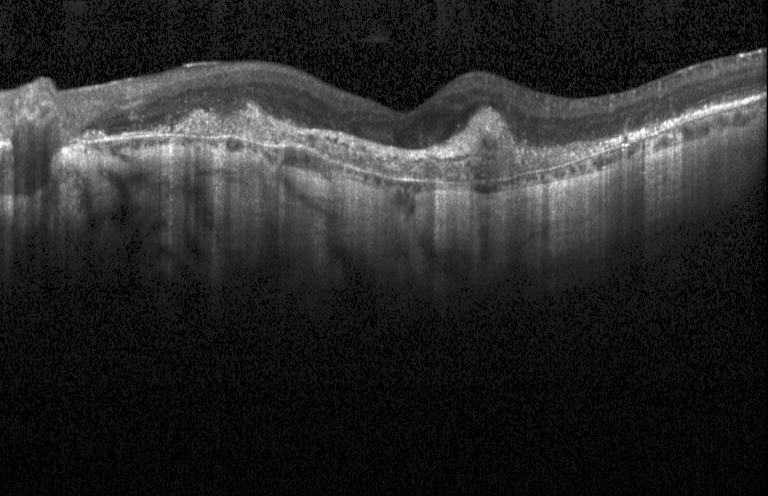 Retinal OCT cross-section.
Choroidal neovascularization.